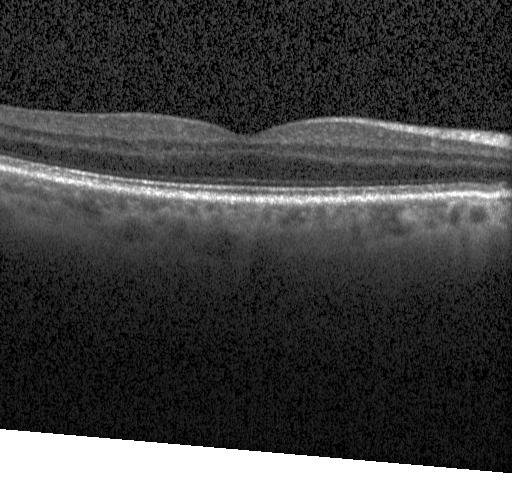 Centered on the fovea · instrument: Heidelberg Spectralis · retinal OCT cross-section. Finding: no evidence of choroidal neovascularization, diabetic macular edema, or drusen.